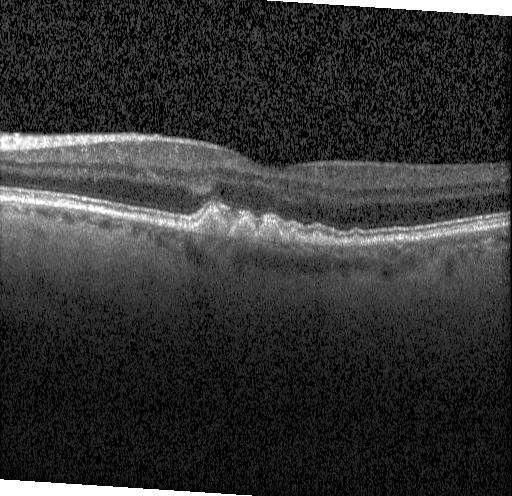 Horizontal scan through the fovea; retinal OCT cross-section — Dx: multiple drusen.